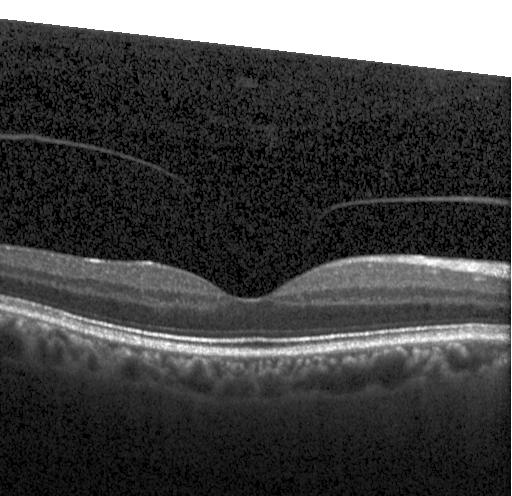

Retinal OCT cross-section showing no evidence of CNV, DME, or drusen.